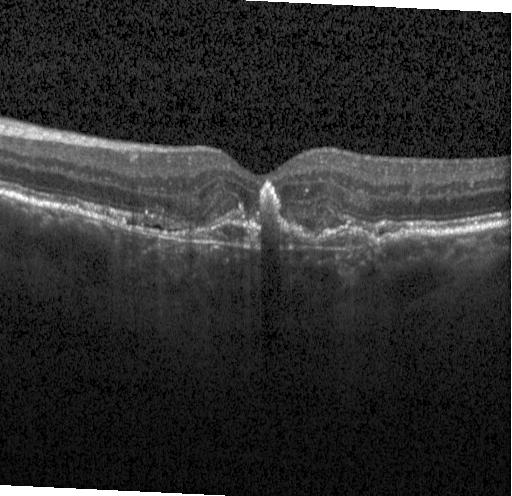

The scan shows choroidal neovascularization.